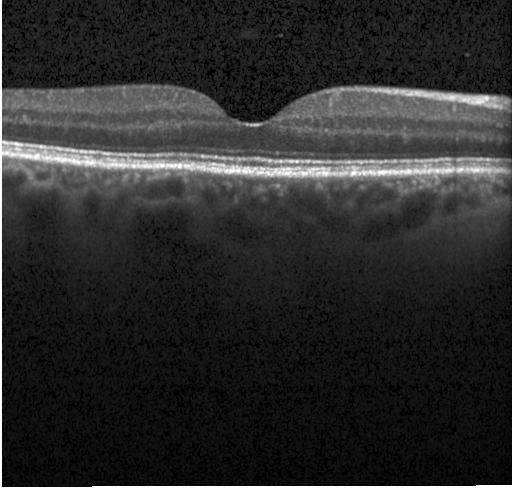

SD-OCT. OCT B-scan
Macular OCT: no CNV, DME, or drusen.